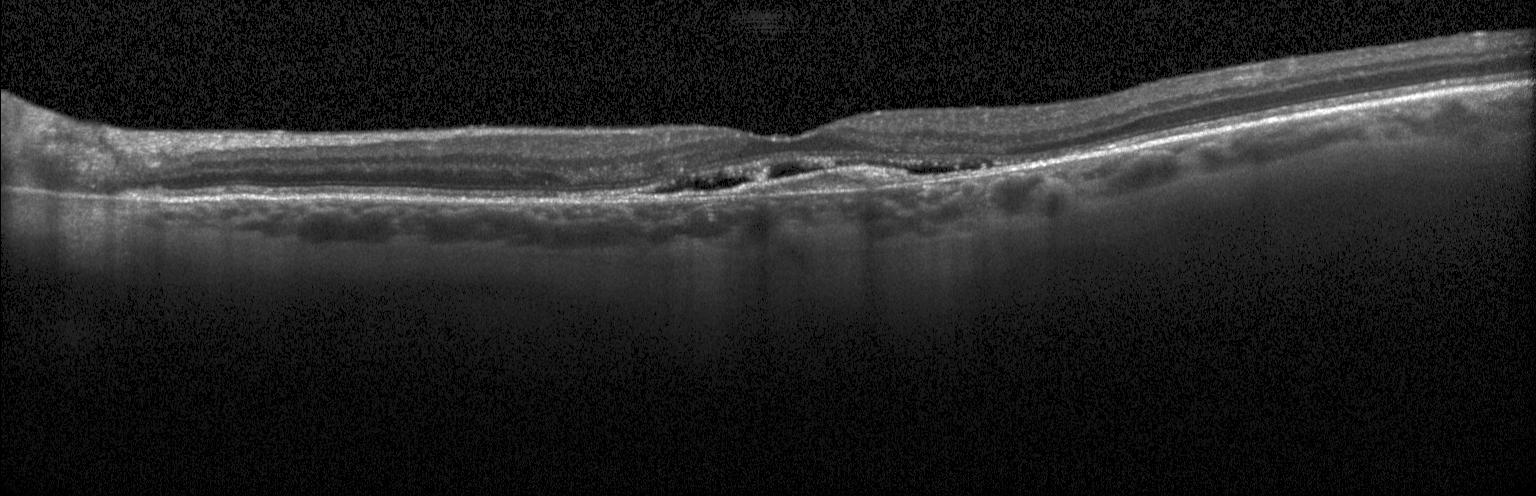

Through the macula. OCT line scan. Diagnosis: a choroidal neovascular membrane.